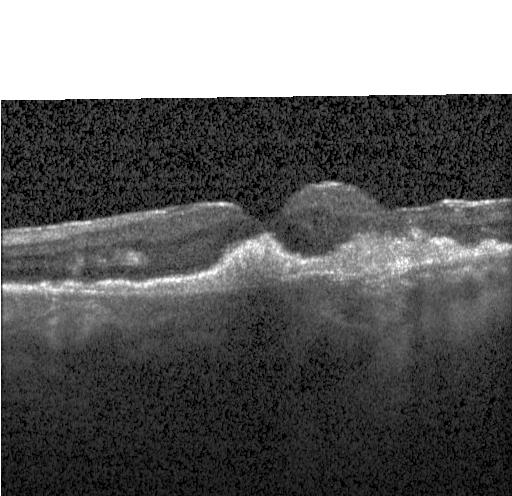 Finding: a choroidal neovascular membrane.